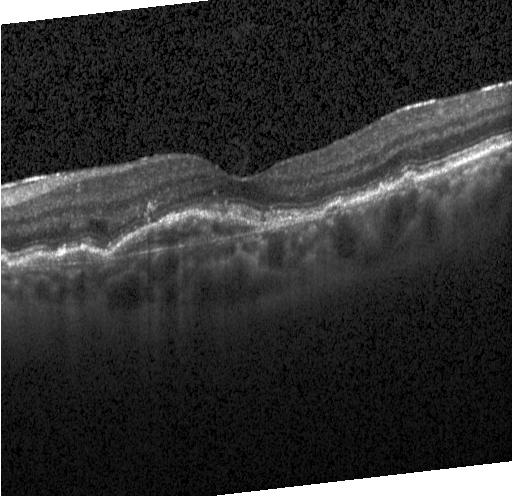
Spectral-domain optical coherence tomography; retinal OCT B-scan; through the macula — Impression: choroidal neovascularization (CNV).